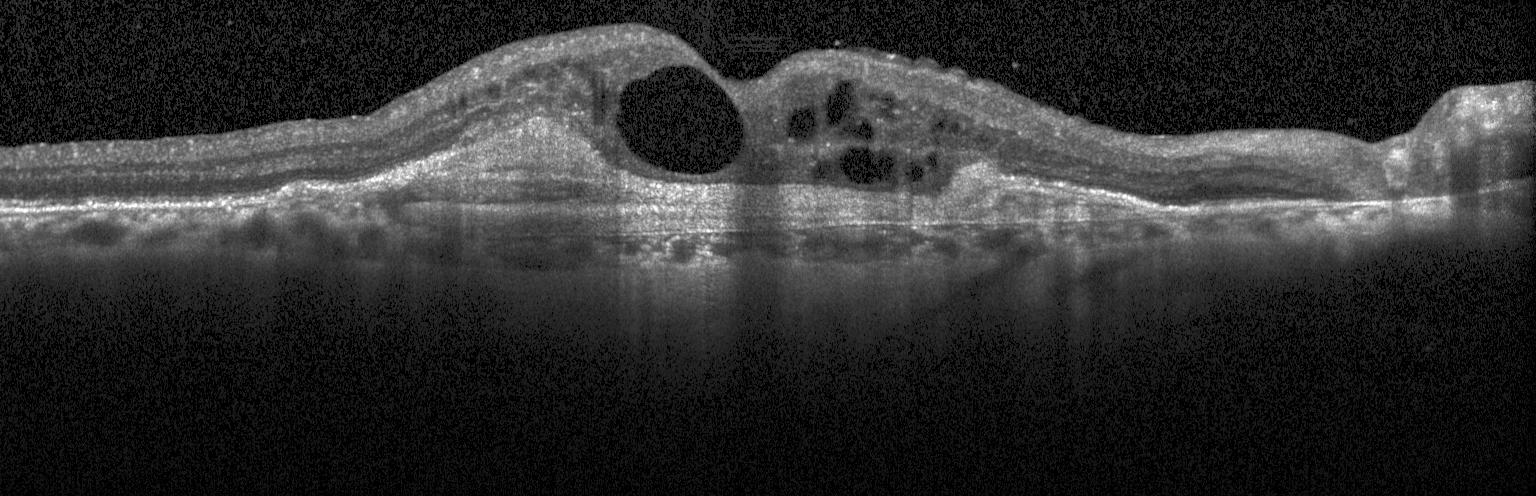
Impression: a choroidal neovascular membrane.